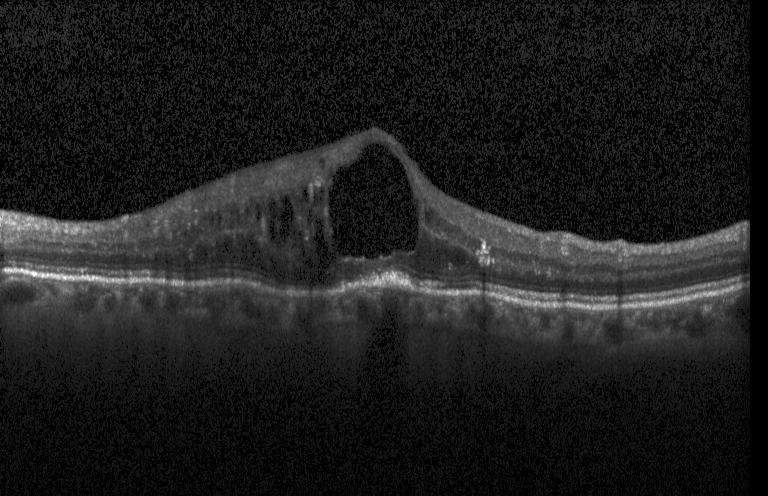 Retinal OCT cross-section. Diagnosis: diabetic macular edema.